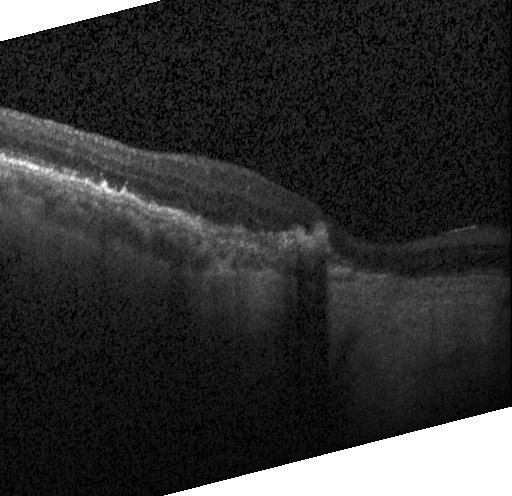
SD-OCT · centered on the fovea · retinal OCT cross-section · Heidelberg Spectralis
Diagnosis: a choroidal neovascular membrane.